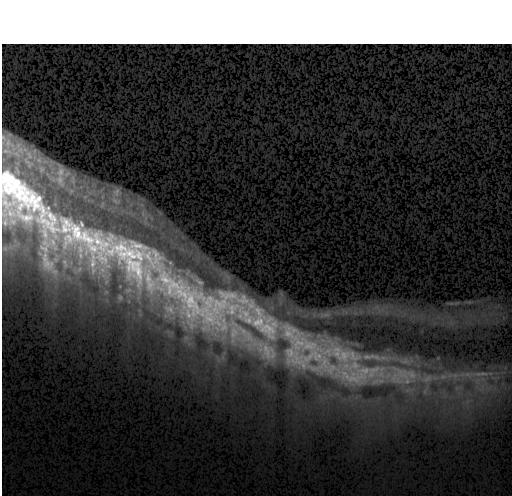

OCT line scan. Diagnosis: choroidal neovascularization.